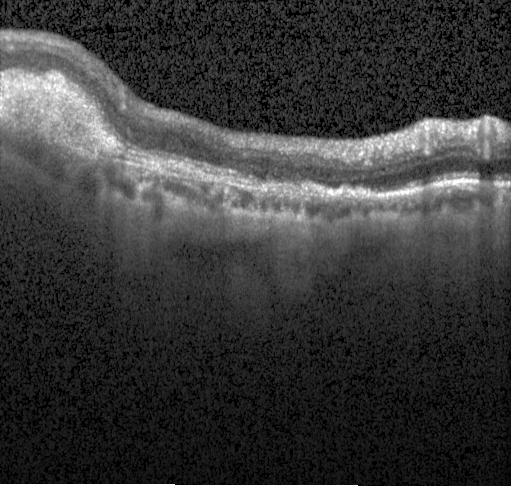 The scan shows choroidal neovascularization.